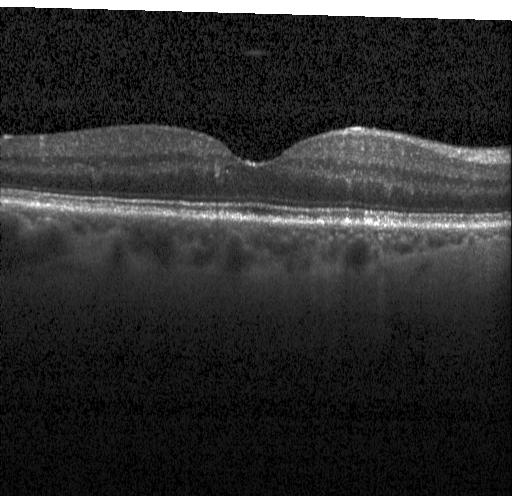 OCT B-scan.
Finding: no choroidal neovascularization, diabetic macular edema, or drusen.